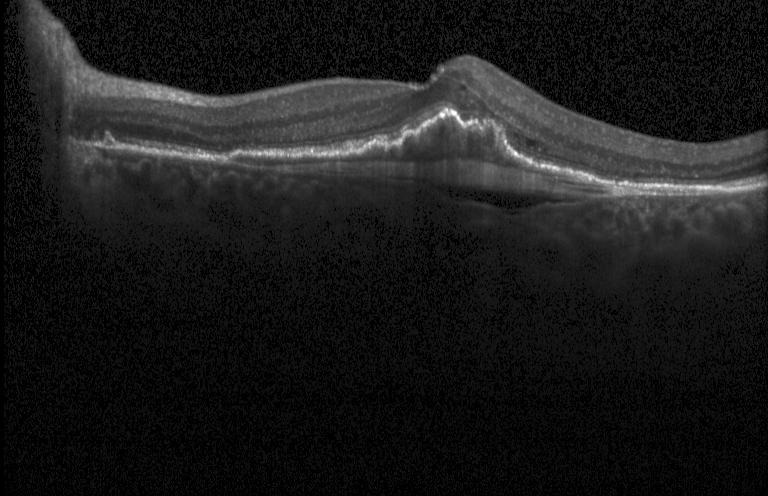

Optical coherence tomography scan; through the macula; acquired on a Heidelberg Spectralis
The scan shows CNV.